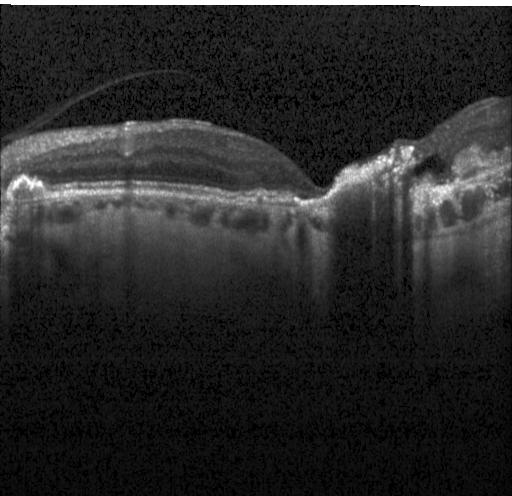
Optical coherence tomography scan. Horizontal scan through the fovea.
Assessment: a choroidal neovascular membrane.